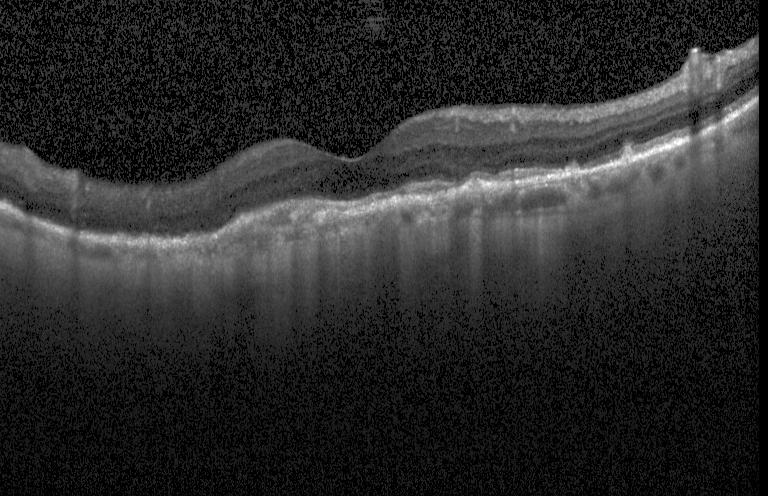

Macular OCT demonstrating CNV.